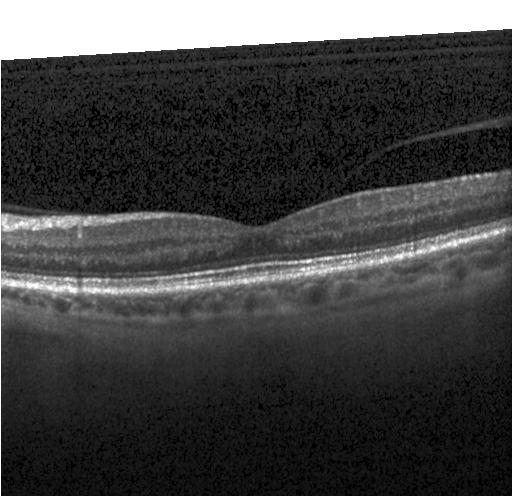

Finding: no CNV, DME, or drusen.